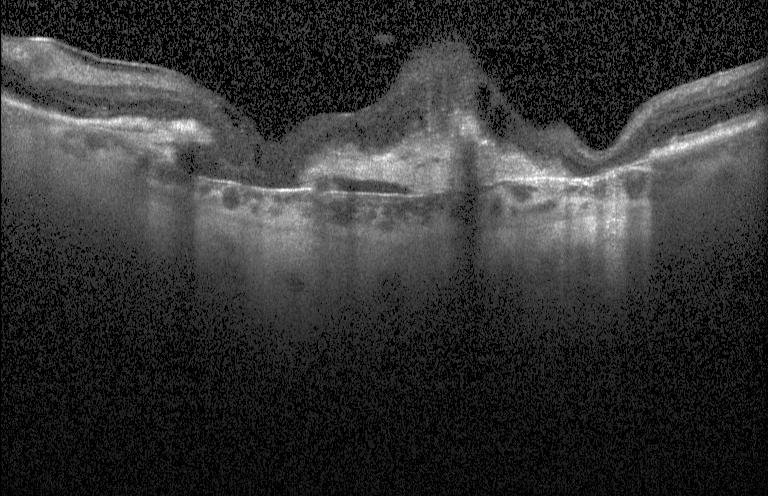

Retinal OCT cross-section showing choroidal neovascularization.